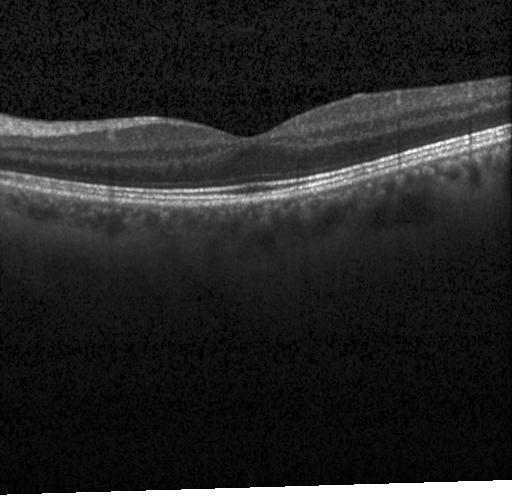

Dx: no choroidal neovascularization, no diabetic macular edema, and no drusen.